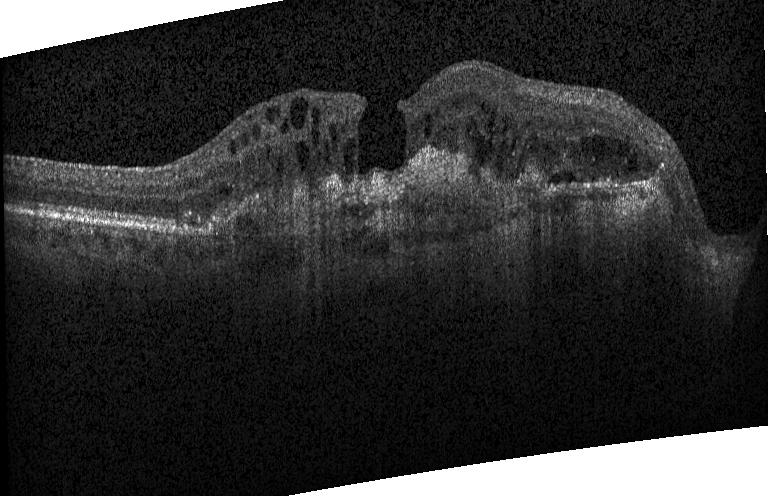 Acquired on a Heidelberg Spectralis, optical coherence tomography scan, SD-OCT — The scan shows a choroidal neovascular membrane.